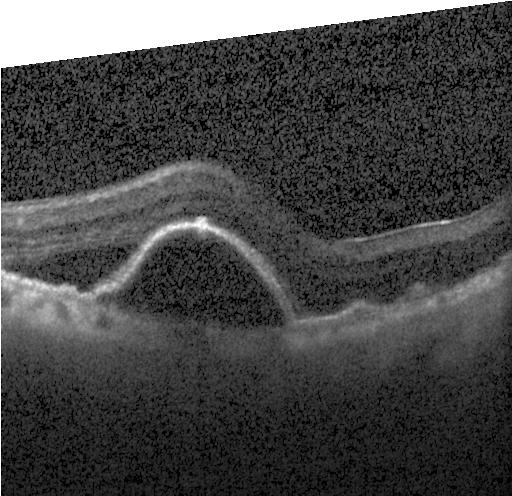
Heidelberg Spectralis OCT system · retinal OCT B-scan · macular scan · spectral-domain OCT.
A choroidal neovascular membrane.